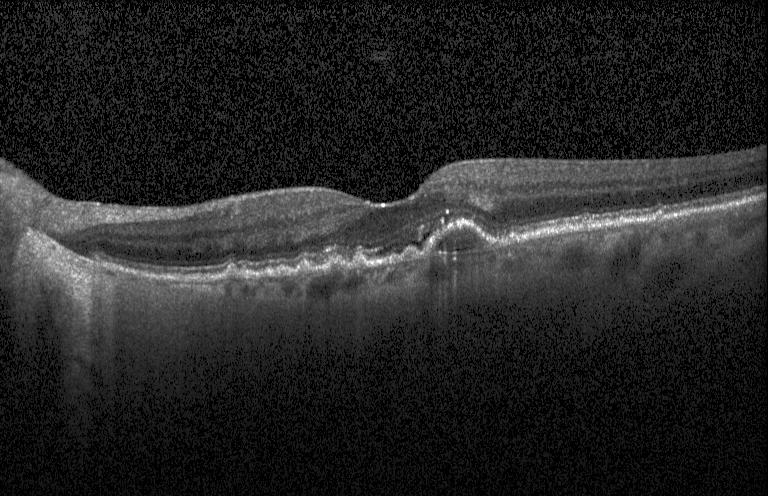
Optical coherence tomography scan — This B-scan demonstrates a choroidal neovascular membrane.